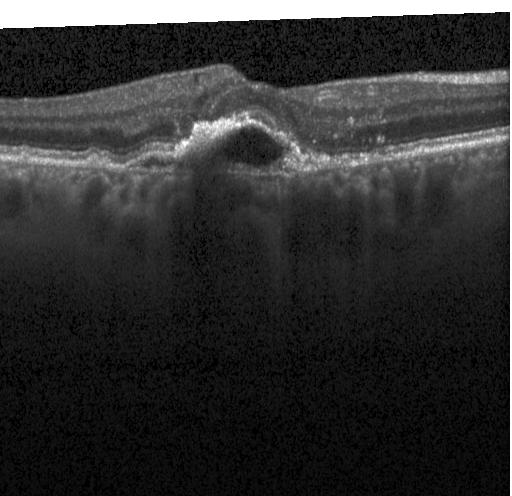
Horizontal scan through the fovea. Spectral-domain OCT. Acquired on a Heidelberg Spectralis. Retinal OCT cross-section. OCT finding: CNV.